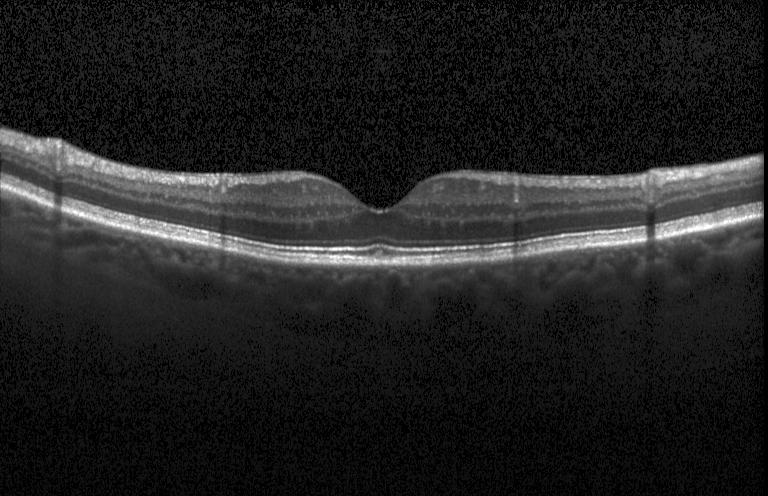

OCT line scan; instrument: Heidelberg Spectralis.
Impression: neither choroidal neovascularization, diabetic macular edema, nor drusen.